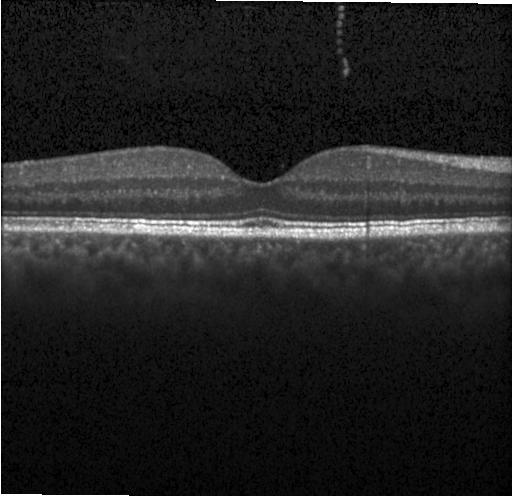 The scan shows no choroidal neovascularization, diabetic macular edema, or drusen.